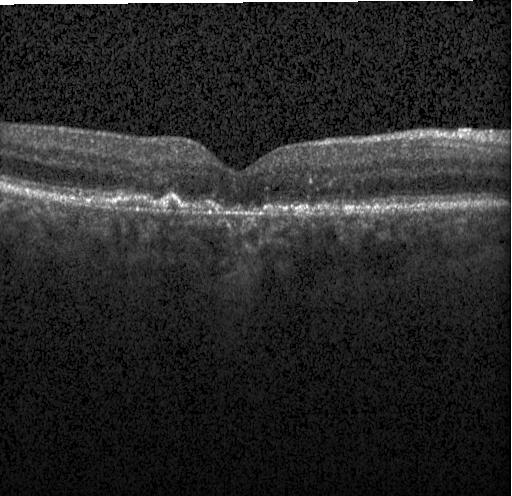

OCT finding: choroidal neovascularization (CNV).